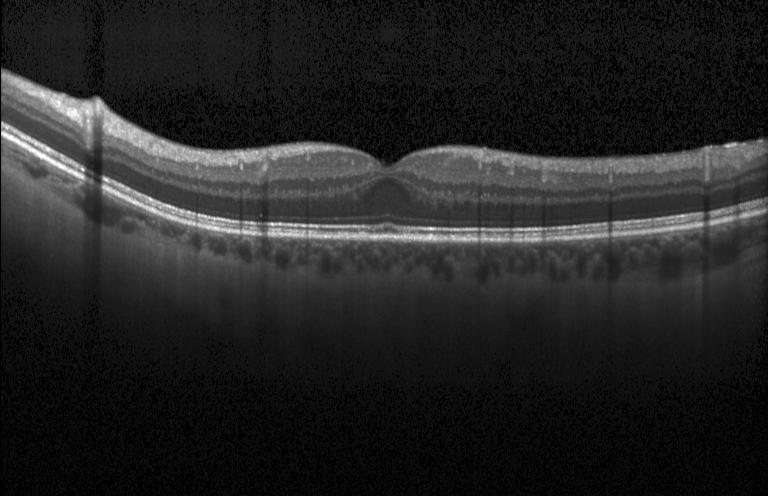
Instrument: Heidelberg Spectralis. Fovea-centered. Spectral-domain optical coherence tomography. Retinal OCT cross-section. Finding: no choroidal neovascularization, diabetic macular edema, or drusen.